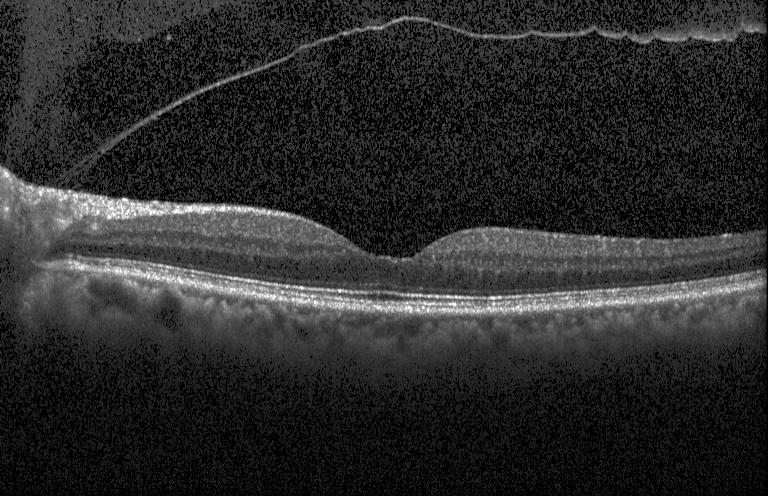 Heidelberg Spectralis · fovea-centered · retinal OCT cross-section · SD-OCT — Diagnosis: no choroidal neovascularization, no diabetic macular edema, and no drusen.